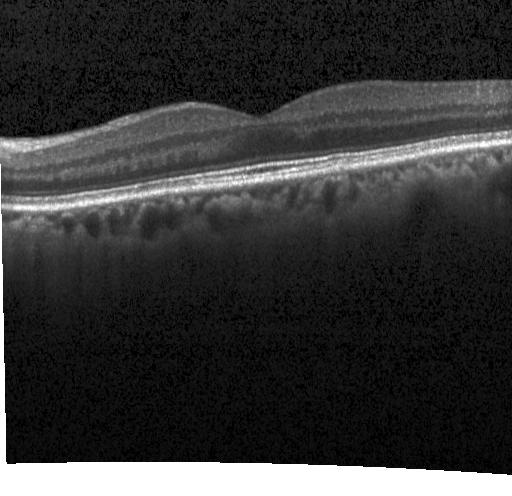
Finding: no choroidal neovascularization, no diabetic macular edema, and no drusen.